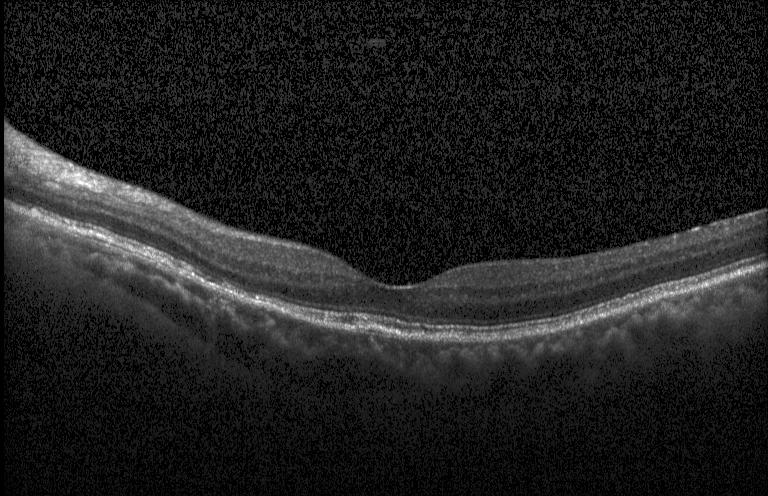 Horizontal scan through the fovea · retinal OCT B-scan · Heidelberg Spectralis · spectral-domain OCT.
The scan shows no choroidal neovascularization, no diabetic macular edema, and no drusen.